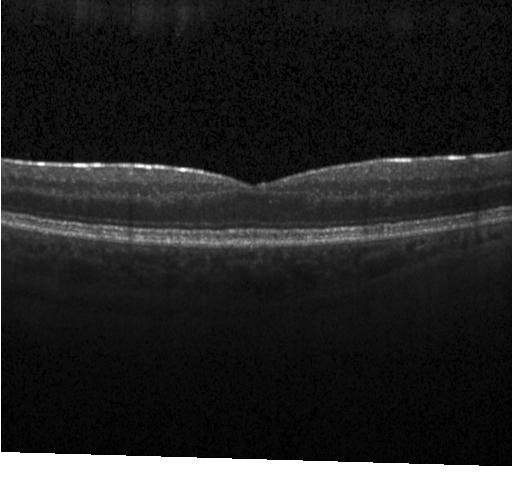 OCT scan showing no choroidal neovascularization, no diabetic macular edema, and no drusen.